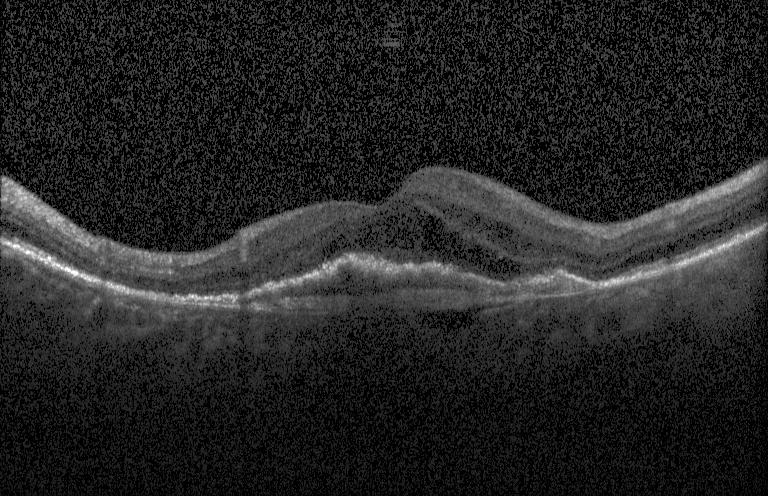 Macular OCT: choroidal neovascularization (CNV).